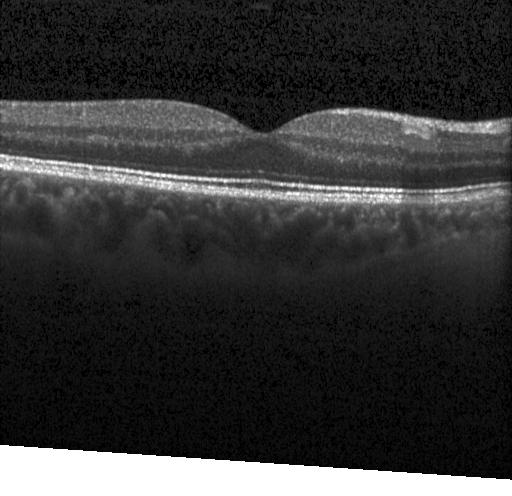

Diagnosis: neither choroidal neovascularization, diabetic macular edema, nor drusen.